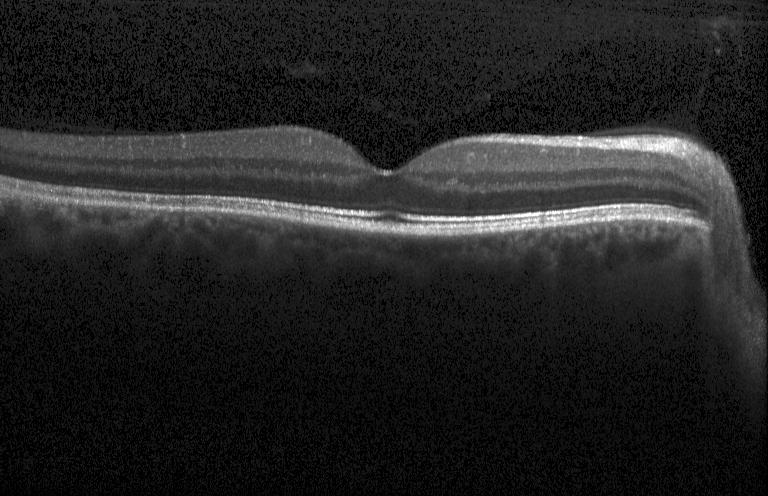

Diagnosis: no evidence of CNV, DME, or drusen.